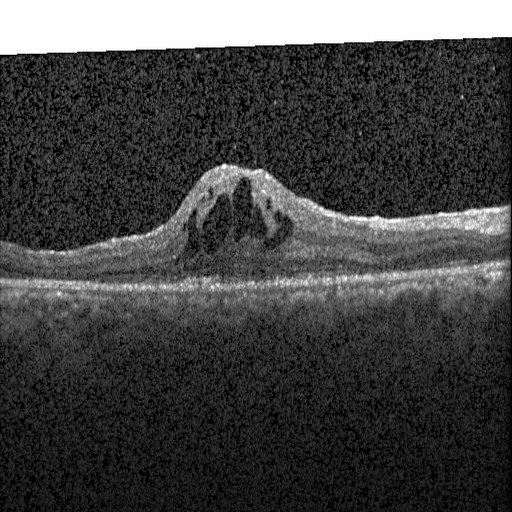

OCT scan showing DME.